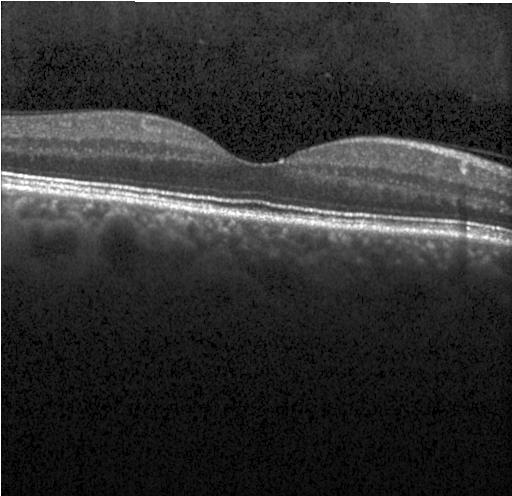
OCT line scan — Diagnosis: no choroidal neovascularization, diabetic macular edema, or drusen.